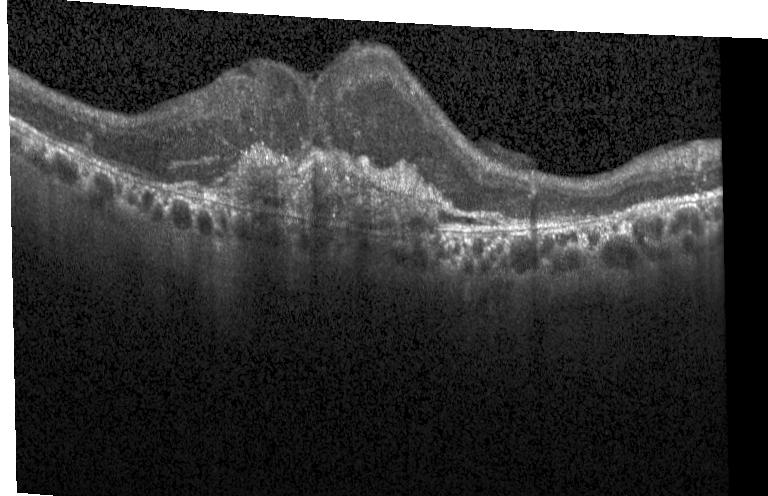 Finding: a choroidal neovascular membrane.